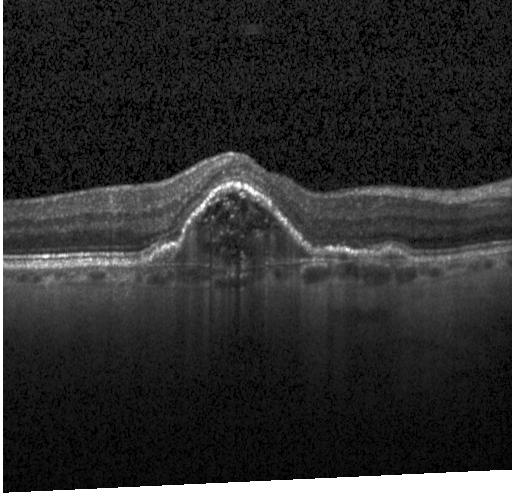

Spectral-domain OCT · OCT B-scan · macular scan.
Impression: choroidal neovascularization (CNV).